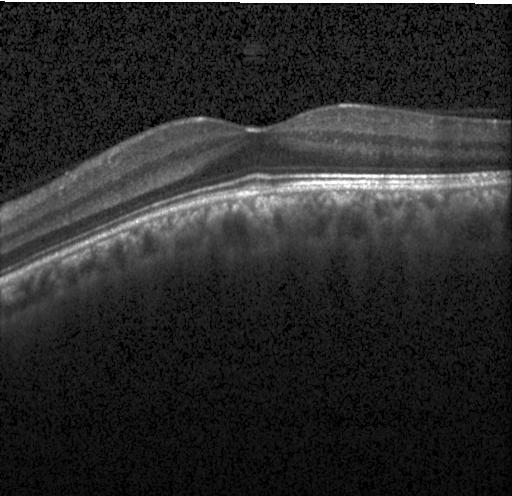
Retinal OCT B-scan. OCT finding: no CNV, no DME, and no drusen.